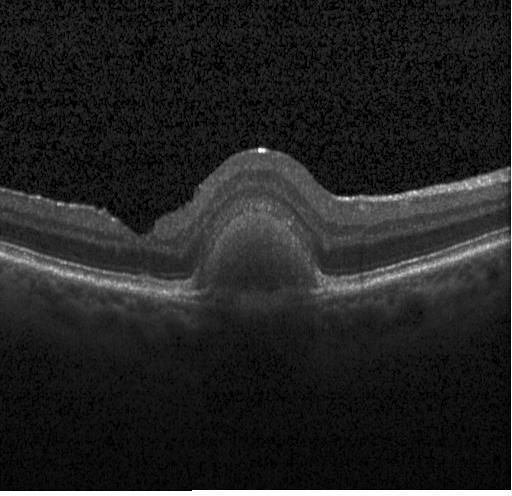

OCT B-scan, SD-OCT
Finding: CNV.